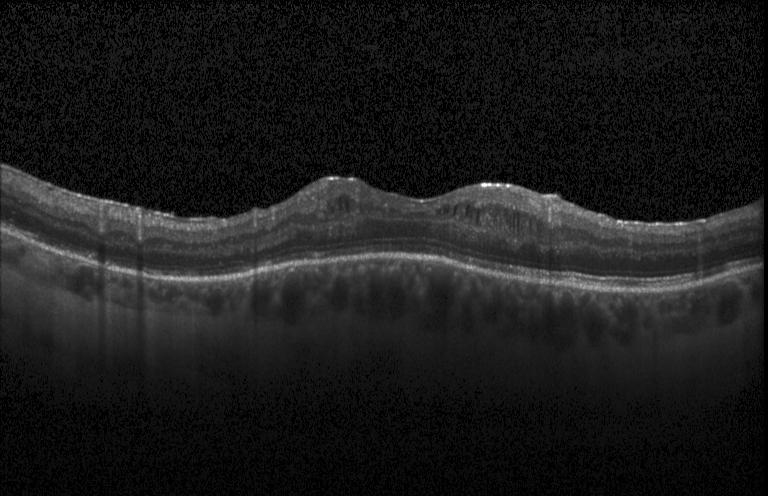
Impression: diabetic macular edema.